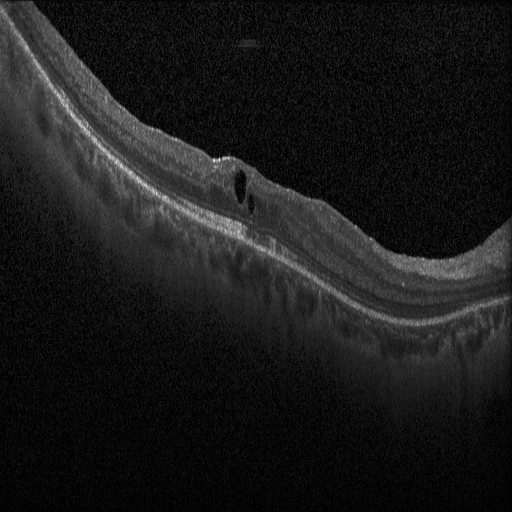 Diagnosis: diabetic macular edema (DME).